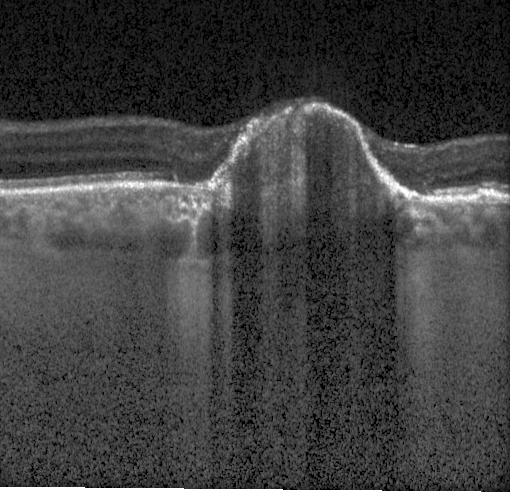
Optical coherence tomography B-scan; SD-OCT.
Impression: a choroidal neovascular membrane.